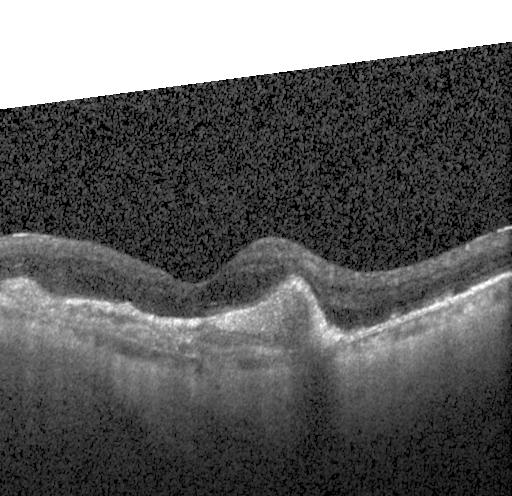

OCT B-scan showing a choroidal neovascular membrane.